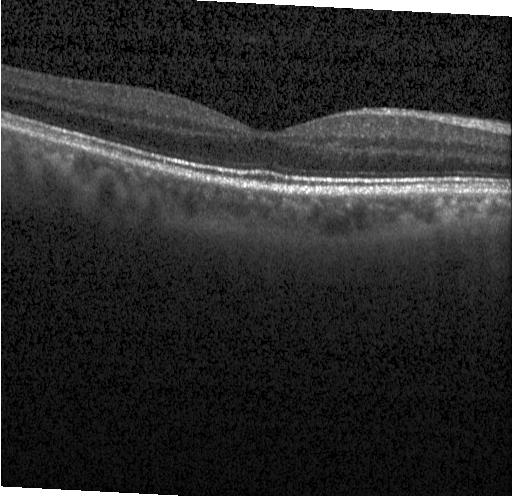

Retinal OCT cross-section. Impression: no evidence of choroidal neovascularization, diabetic macular edema, or drusen.